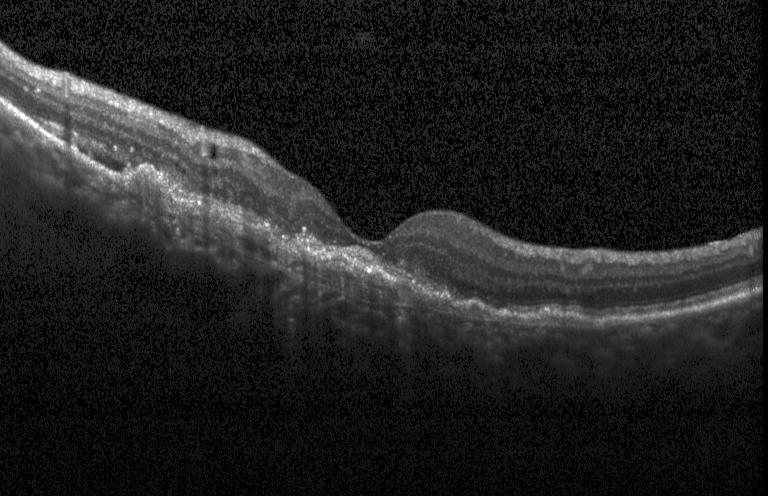

Spectral-domain OCT. Retinal OCT cross-section
Macular OCT: a choroidal neovascular membrane.